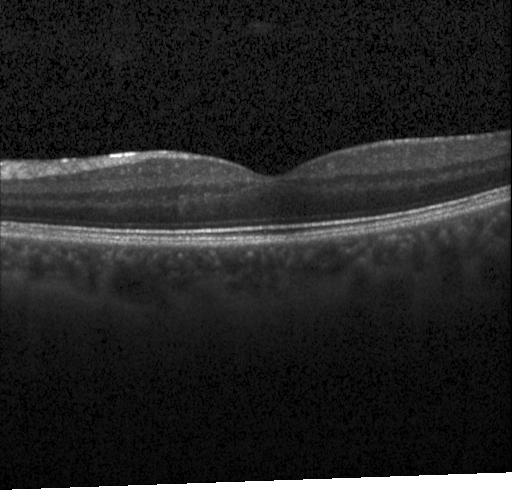

Optical coherence tomography scan; SD-OCT.
Diagnosis: no evidence of choroidal neovascularization, diabetic macular edema, or drusen.